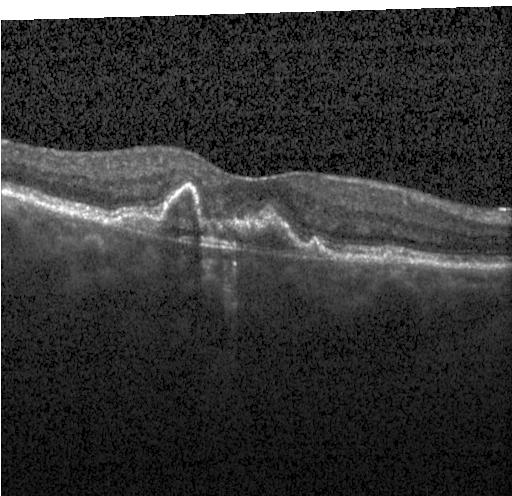 Centered on the fovea, OCT line scan, spectral-domain optical coherence tomography
This B-scan demonstrates a choroidal neovascular membrane.